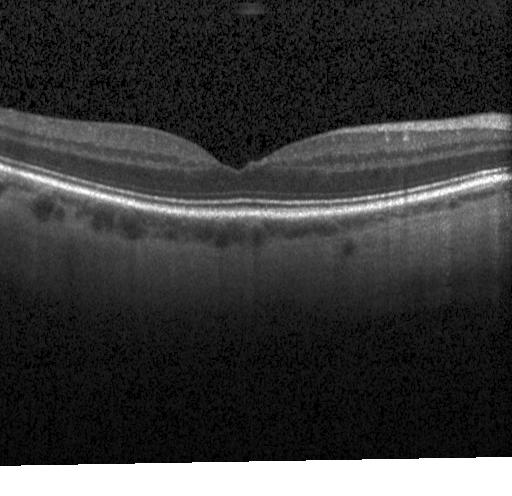
Heidelberg Spectralis. OCT B-scan. Fovea-centered. Finding: no choroidal neovascularization, diabetic macular edema, or drusen.